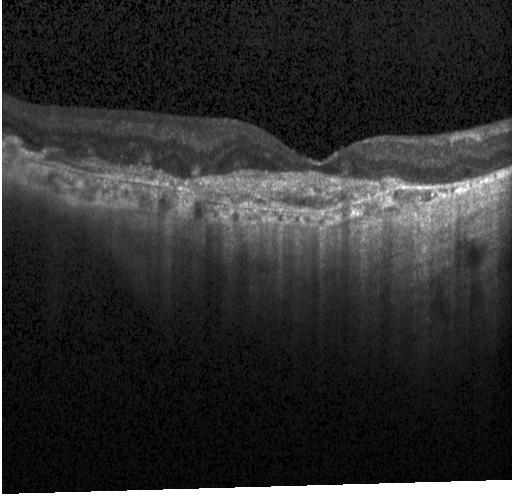 Instrument: Heidelberg Spectralis. Retinal OCT B-scan — A choroidal neovascular membrane.